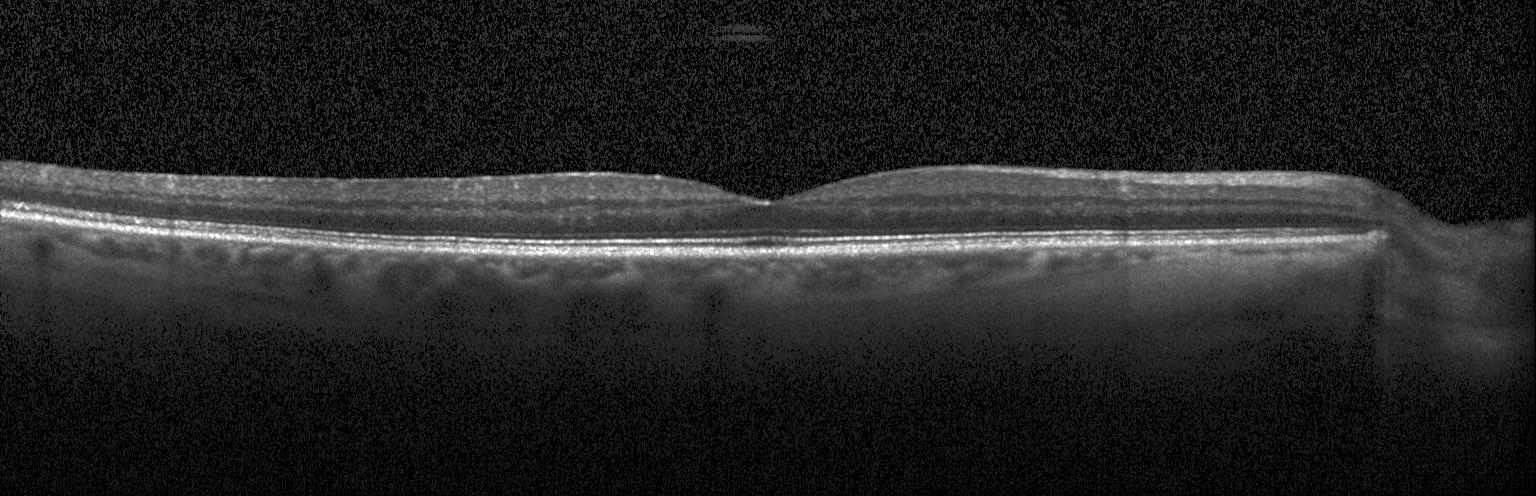

Finding: no evidence of CNV, DME, or drusen.